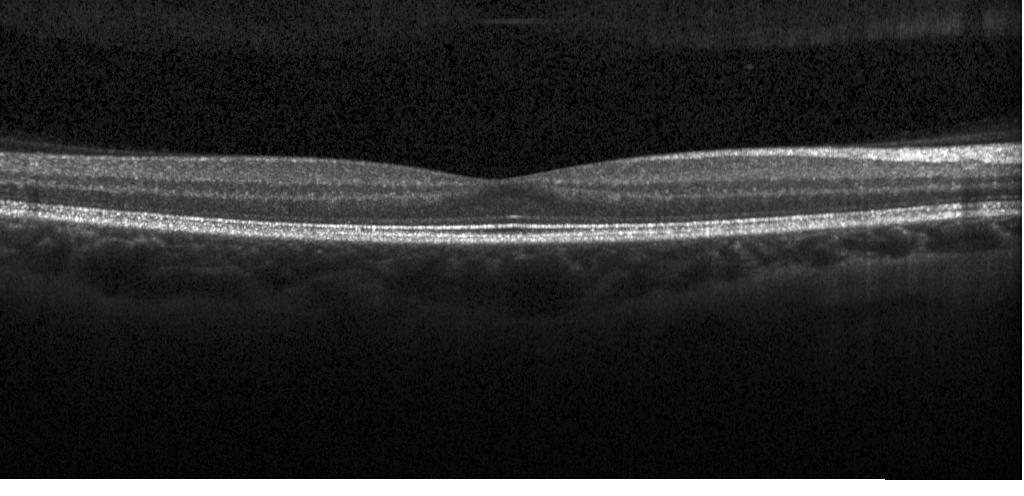
OCT finding: no evidence of choroidal neovascularization, diabetic macular edema, or drusen.